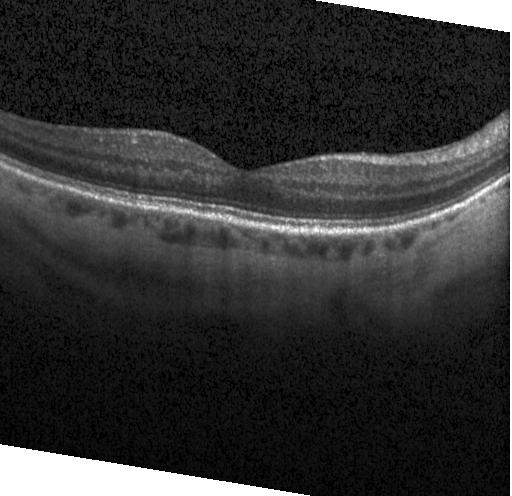 Macular OCT demonstrating neither CNV, DME, nor drusen.